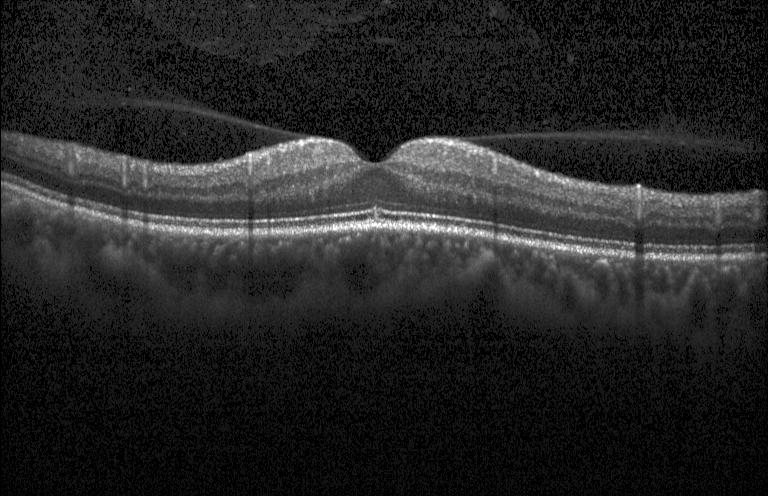
Macular OCT: no CNV, no DME, and no drusen.